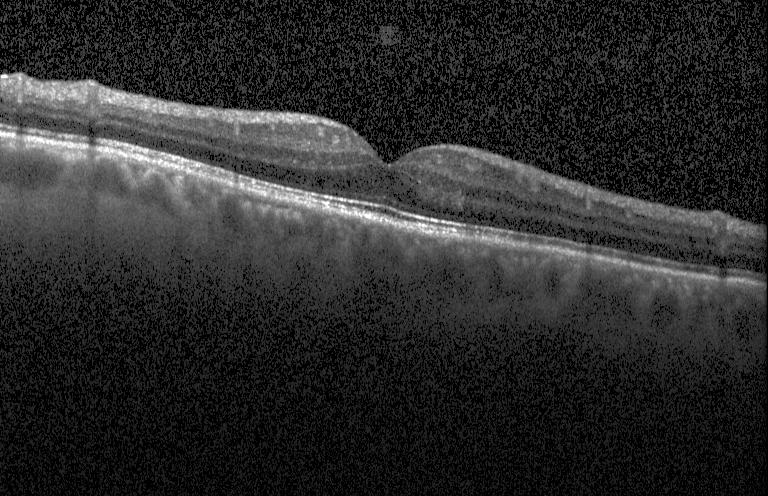

Optical coherence tomography scan, spectral-domain optical coherence tomography, instrument: Heidelberg Spectralis, horizontal scan through the fovea
The scan shows no evidence of choroidal neovascularization, diabetic macular edema, or drusen.